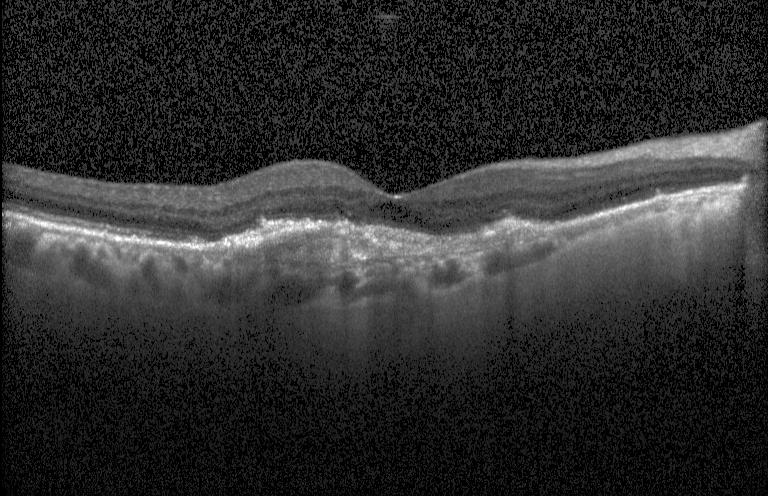 OCT finding: choroidal neovascularization (CNV).